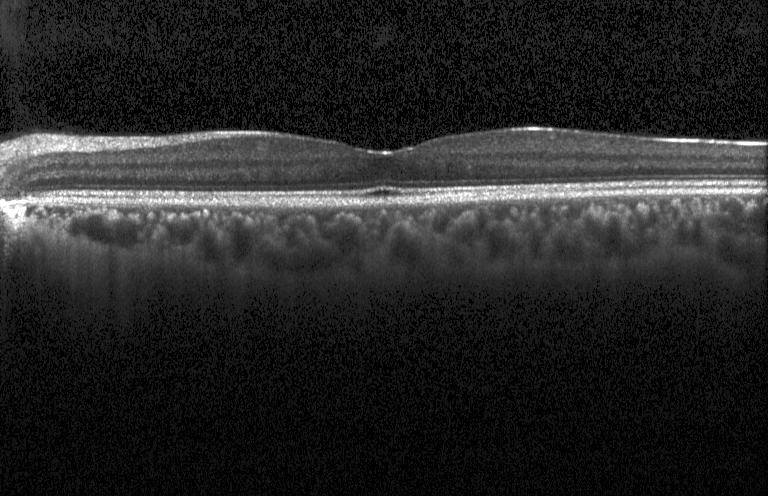

Impression: no choroidal neovascularization, no diabetic macular edema, and no drusen.